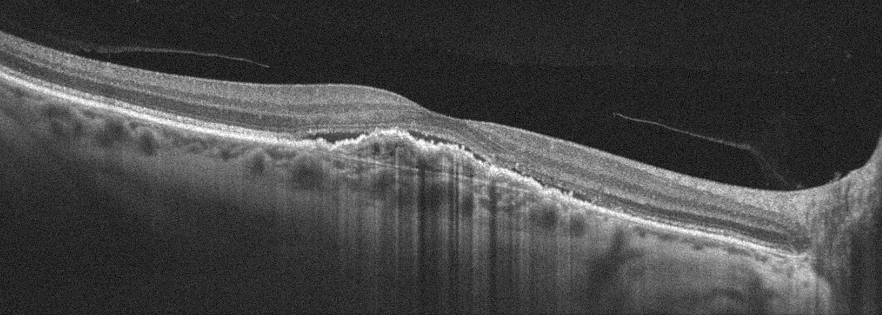

Acquired on an Optovue Avanti RTVue XR · optical coherence tomography scan · fovea-centered.
Impression: age-related macular degeneration (AMD).